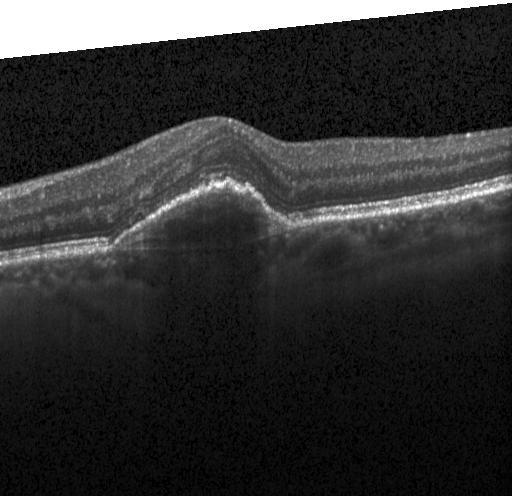
Dx: choroidal neovascularization.